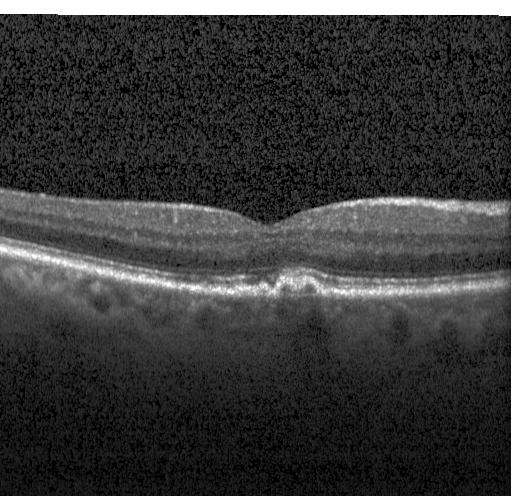

OCT B-scan. Diagnosis: sub-RPE drusenoid deposits.